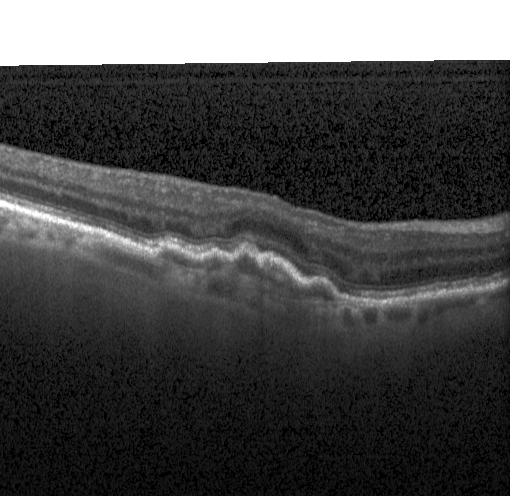 Instrument: Heidelberg Spectralis · macular scan · optical coherence tomography scan · spectral-domain OCT. This B-scan demonstrates a choroidal neovascular membrane.